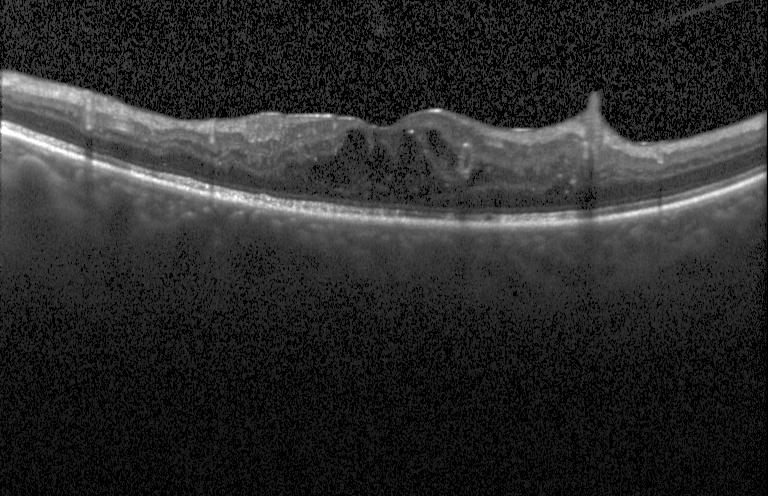
OCT finding: diabetic macular edema (DME).